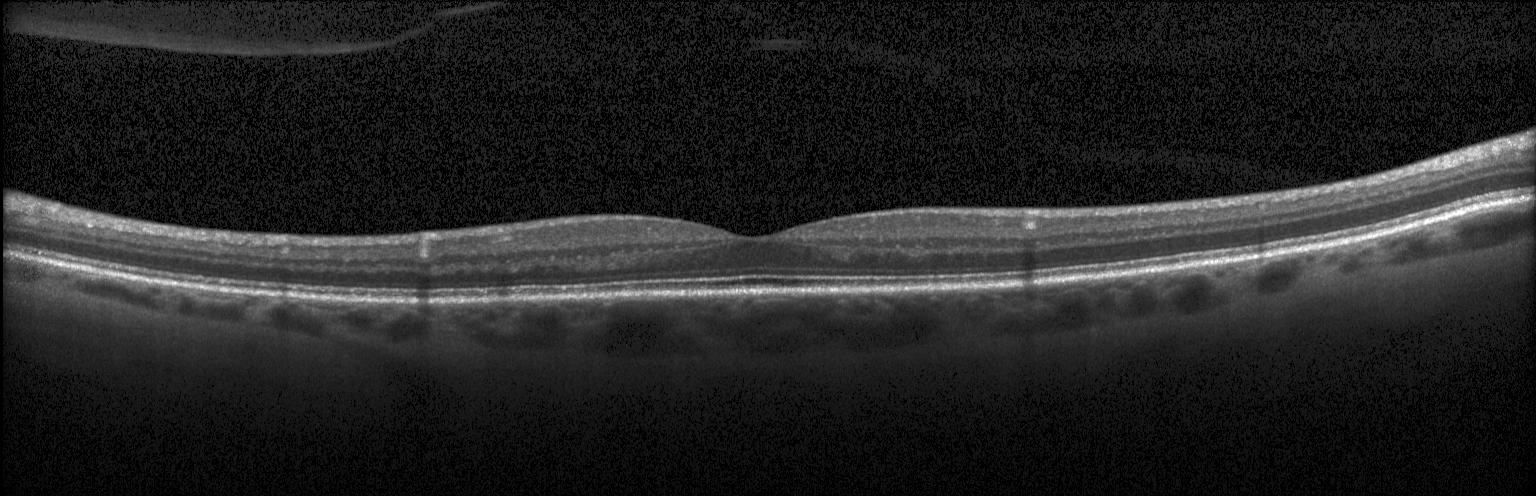

This B-scan demonstrates no choroidal neovascularization, diabetic macular edema, or drusen.